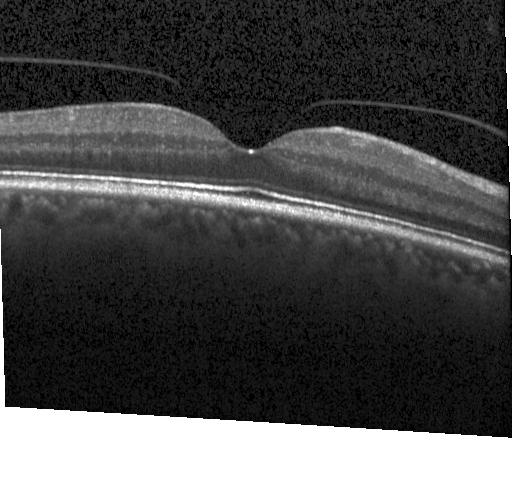
Macular OCT: no choroidal neovascularization, diabetic macular edema, or drusen.